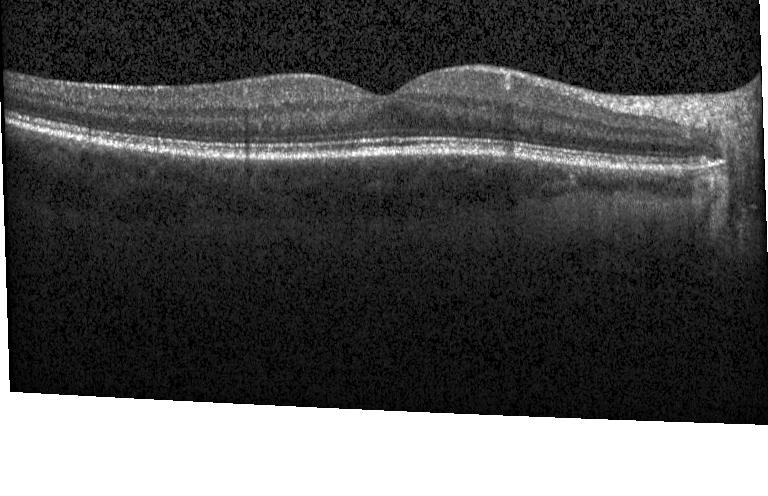

This B-scan demonstrates neither choroidal neovascularization, diabetic macular edema, nor drusen.